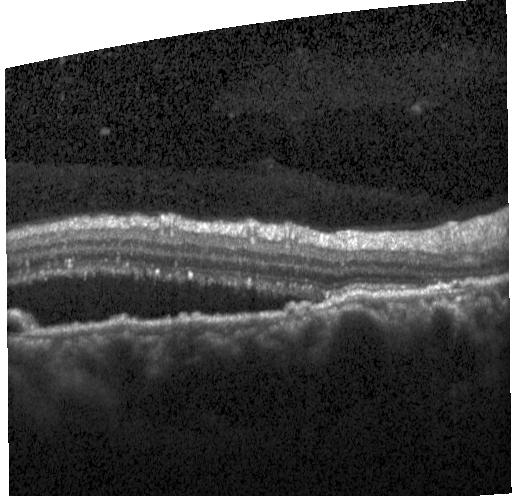

OCT line scan · spectral-domain optical coherence tomography
Assessment: a choroidal neovascular membrane.